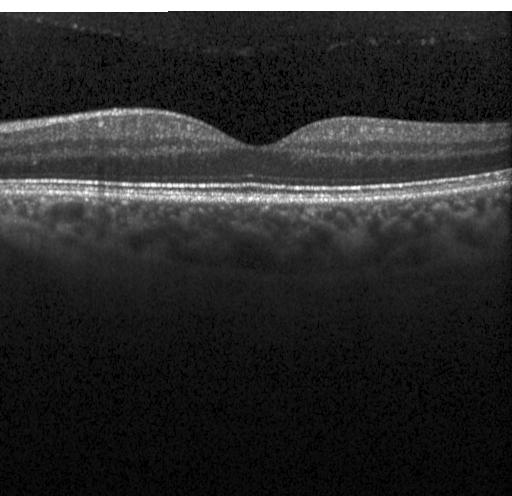
OCT line scan · macular scan · SD-OCT — Diagnosis: no choroidal neovascularization, no diabetic macular edema, and no drusen.